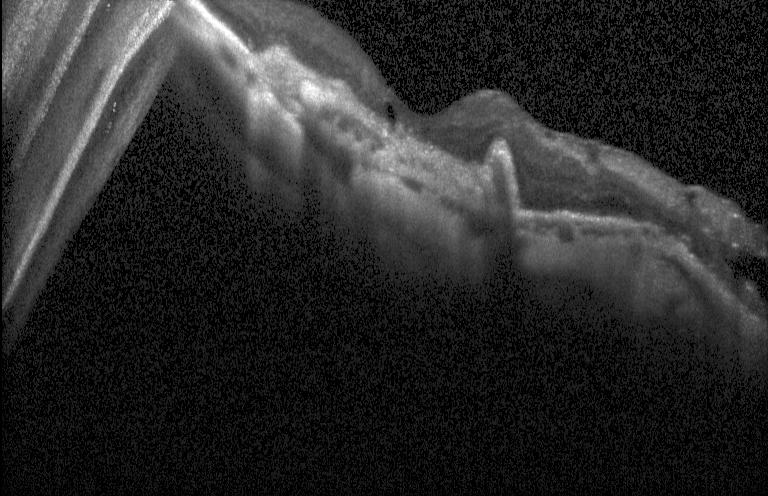 OCT B-scan. Horizontal scan through the fovea — A choroidal neovascular membrane.